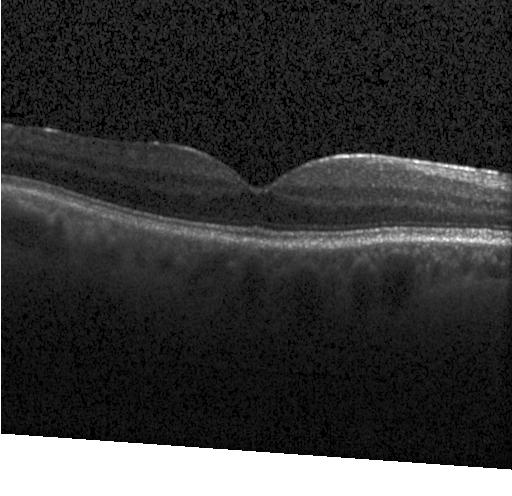 Optical coherence tomography B-scan, spectral-domain optical coherence tomography, Heidelberg Spectralis OCT system
Assessment: no evidence of CNV, DME, or drusen.